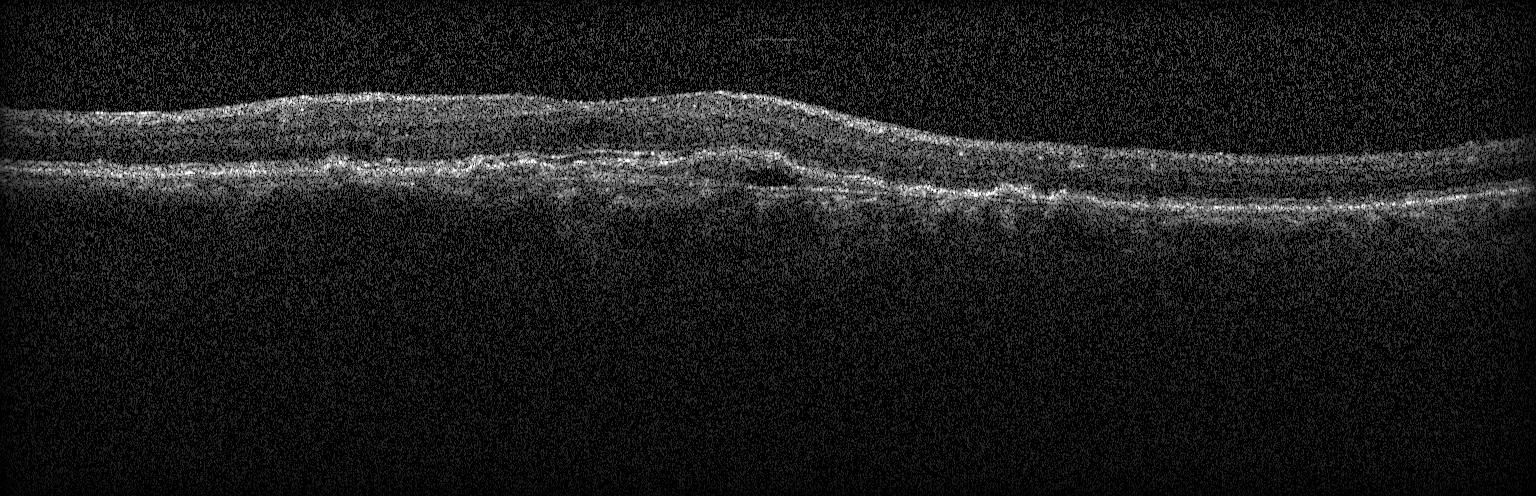
Horizontal scan through the fovea, acquired on a Heidelberg Spectralis, SD-OCT, OCT line scan.
Impression: choroidal neovascularization (CNV).